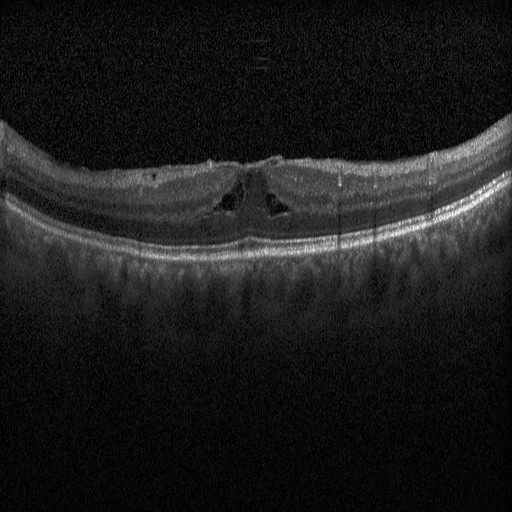 SD-OCT; acquired on a Heidelberg Spectralis; OCT line scan; centered on the fovea — OCT finding: diabetic macular edema (DME).